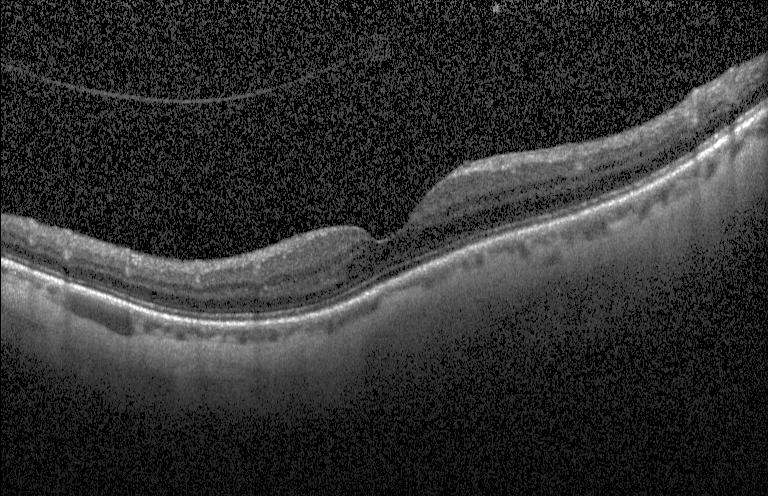

Retinal OCT B-scan. No evidence of choroidal neovascularization, diabetic macular edema, or drusen.